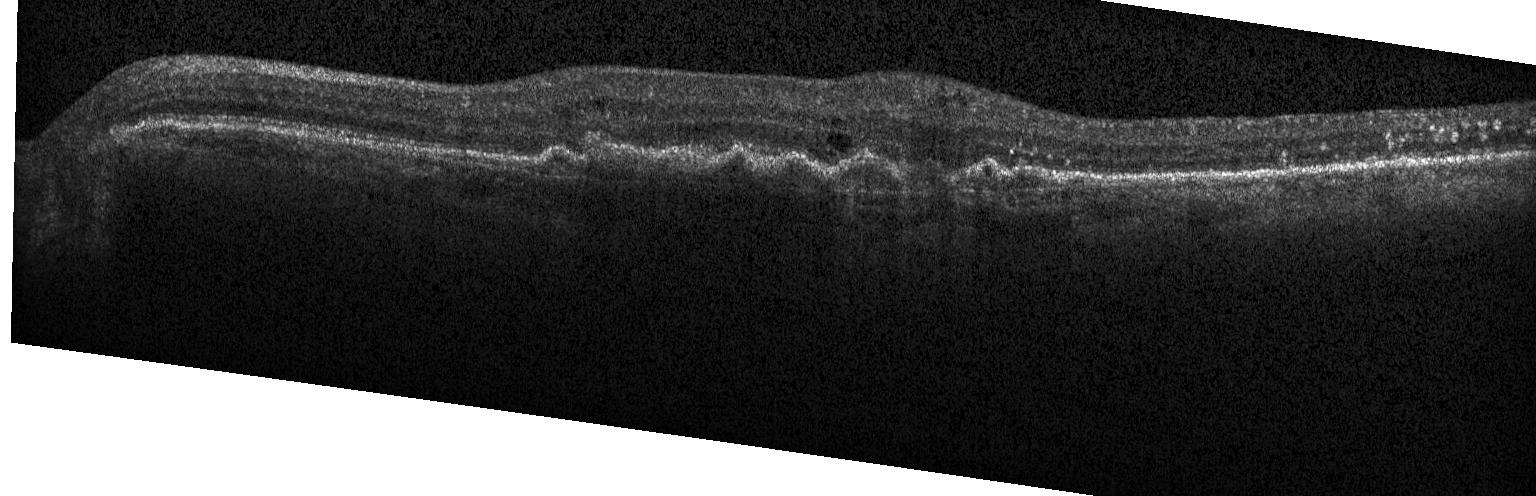

Impression: choroidal neovascularization.